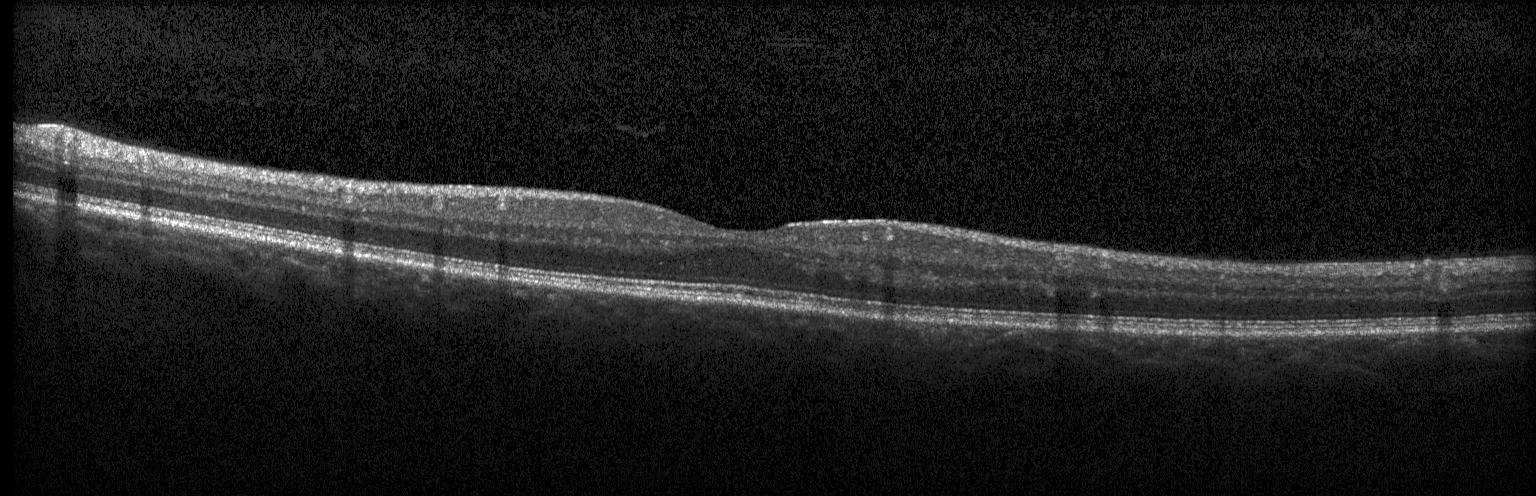

No choroidal neovascularization, diabetic macular edema, or drusen.